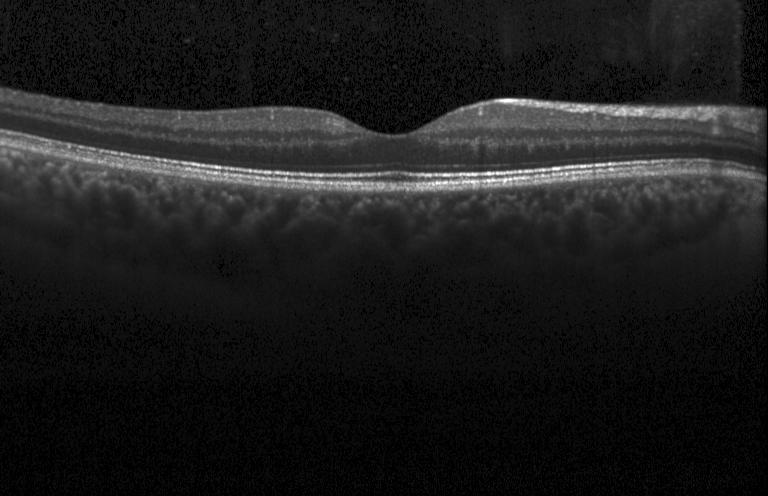

Macular scan. Instrument: Heidelberg Spectralis. Spectral-domain OCT. Optical coherence tomography B-scan — Finding: neither choroidal neovascularization, diabetic macular edema, nor drusen.